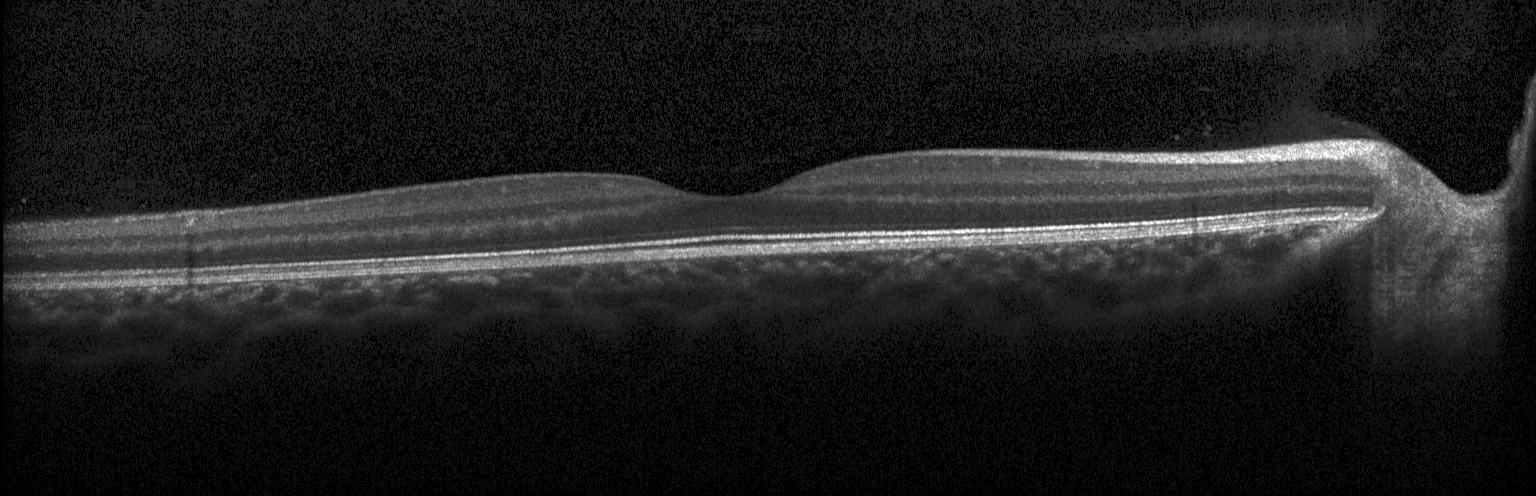
OCT finding: neither choroidal neovascularization, diabetic macular edema, nor drusen.